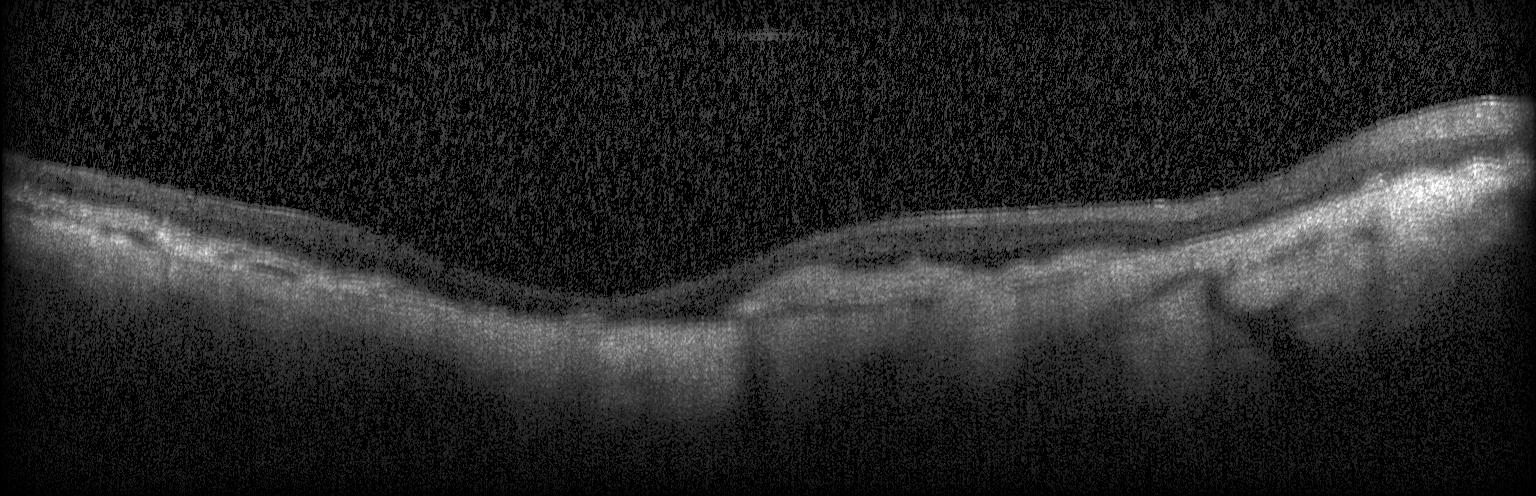 Diagnosis: a choroidal neovascular membrane.